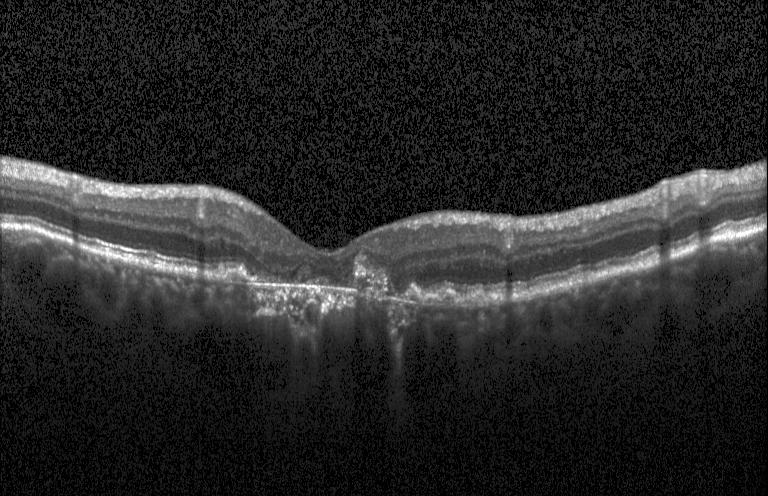

Instrument: Heidelberg Spectralis; macular scan; retinal OCT cross-section; spectral-domain optical coherence tomography
This B-scan demonstrates choroidal neovascularization (CNV).